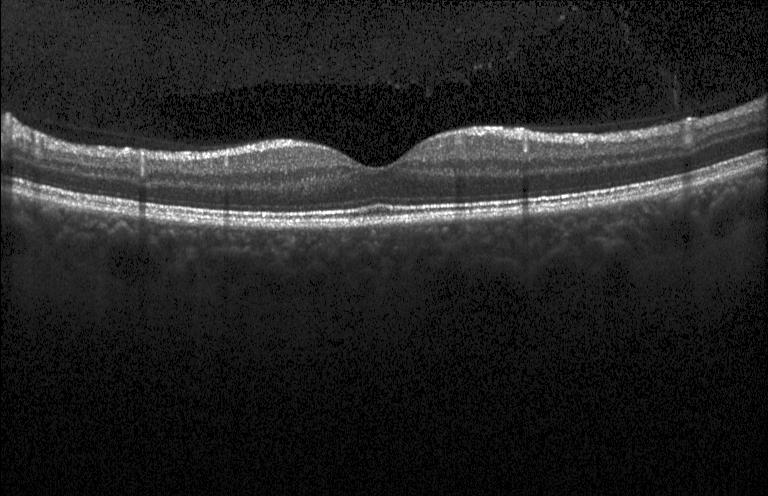
Heidelberg Spectralis OCT system. Through the macula. OCT B-scan. Spectral-domain OCT. Finding: neither choroidal neovascularization, diabetic macular edema, nor drusen.